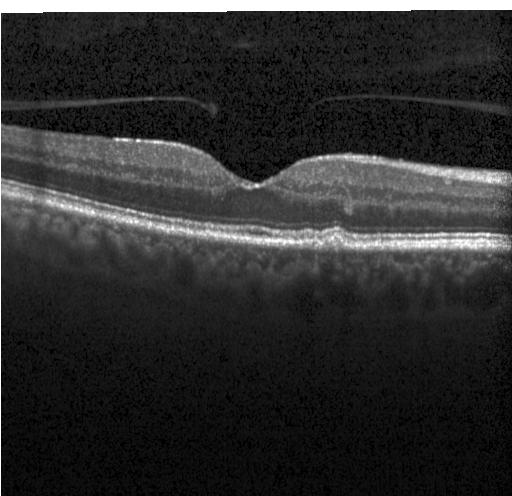
Multiple drusen.